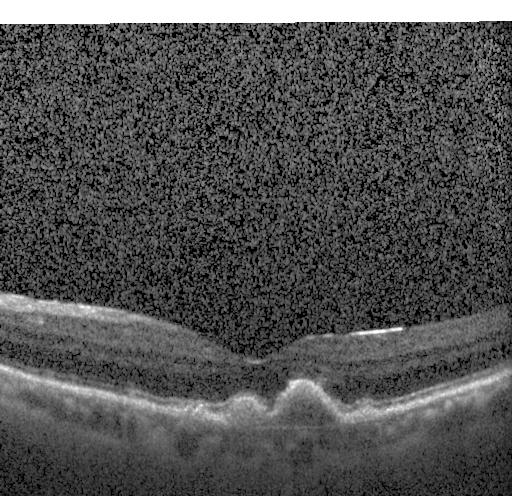
Sub-RPE drusenoid deposits.